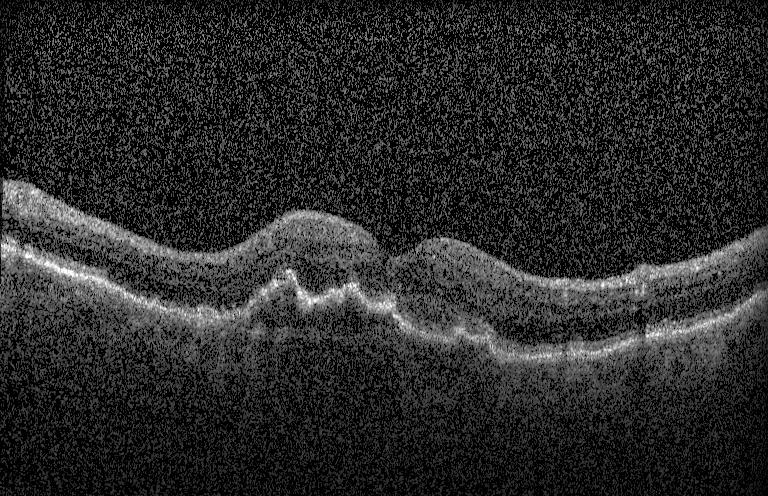 Spectral-domain optical coherence tomography; macular scan; retinal OCT B-scan; instrument: Heidelberg Spectralis.
Assessment: a choroidal neovascular membrane.